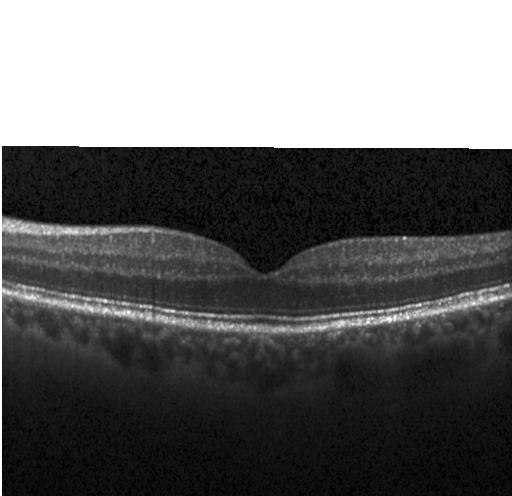 Heidelberg Spectralis. Spectral-domain OCT. Optical coherence tomography scan. Macular scan. This B-scan demonstrates no CNV, DME, or drusen.